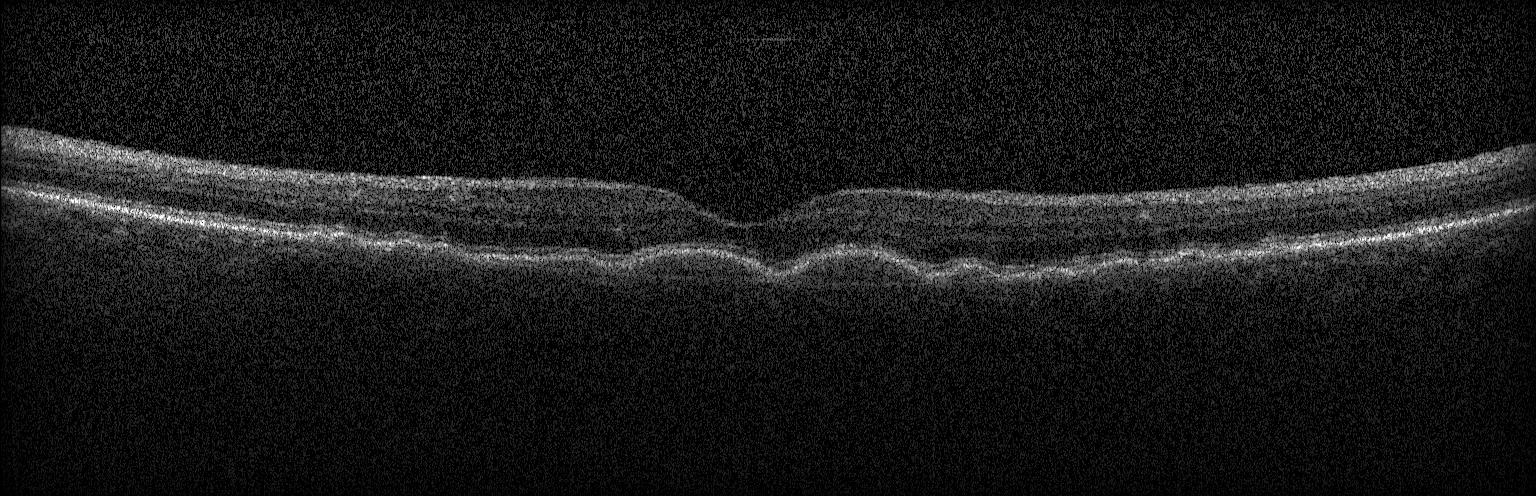

Heidelberg Spectralis OCT system. Retinal OCT cross-section. SD-OCT. Centered on the fovea. Dx: sub-RPE drusenoid deposits.